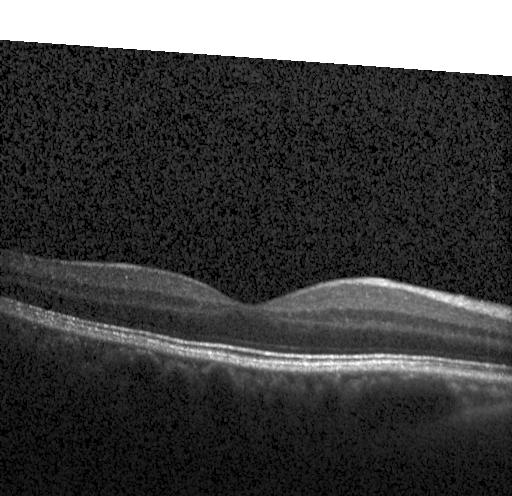 Macular OCT: neither CNV, DME, nor drusen.